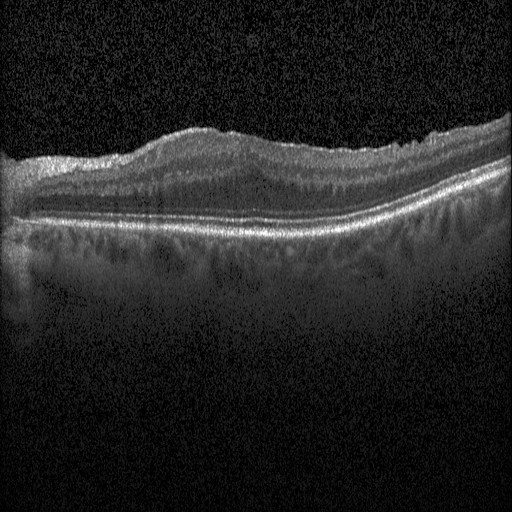 Macular OCT: DME.